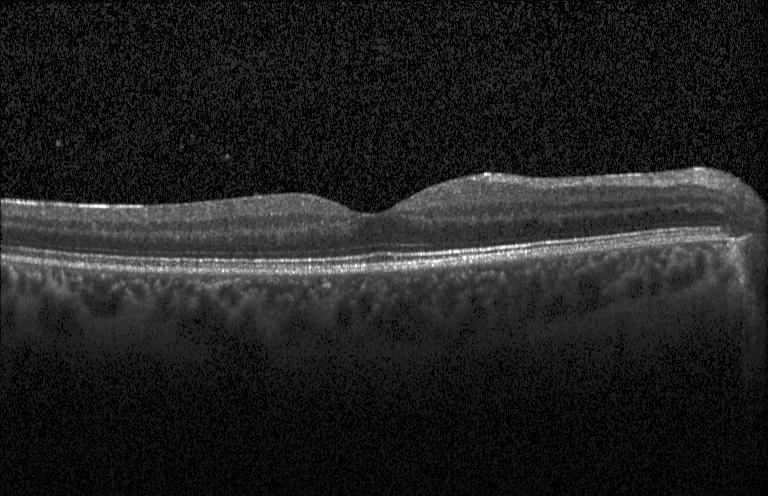 Impression: no choroidal neovascularization, diabetic macular edema, or drusen.